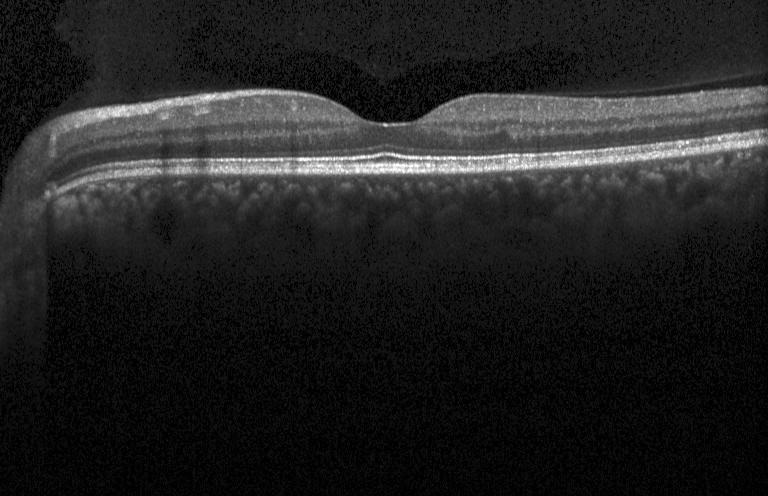 OCT finding: no choroidal neovascularization, diabetic macular edema, or drusen.